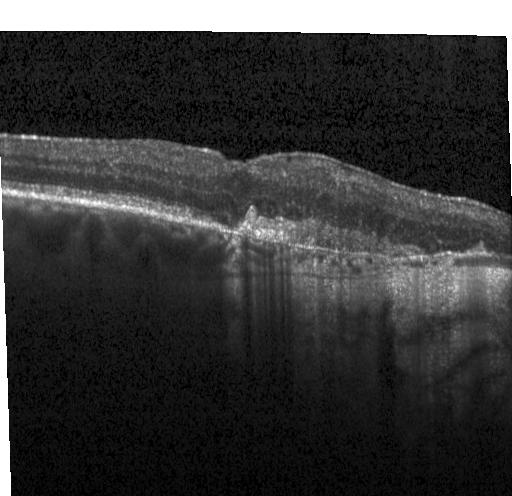 Diagnosis: CNV.